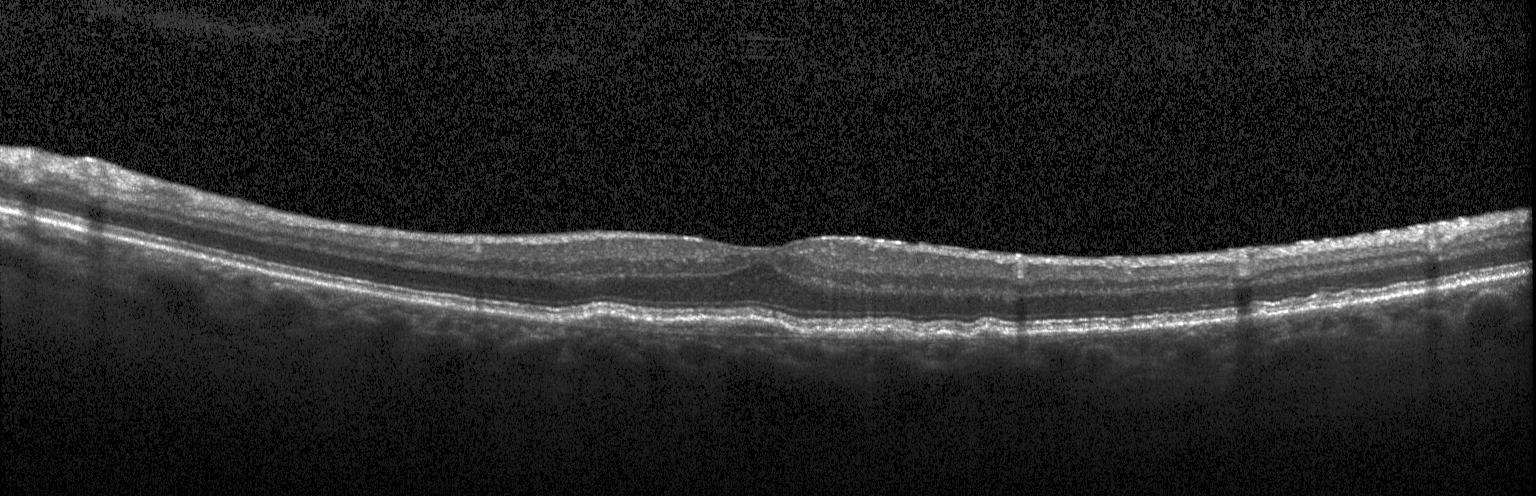 Finding: choroidal neovascularization.